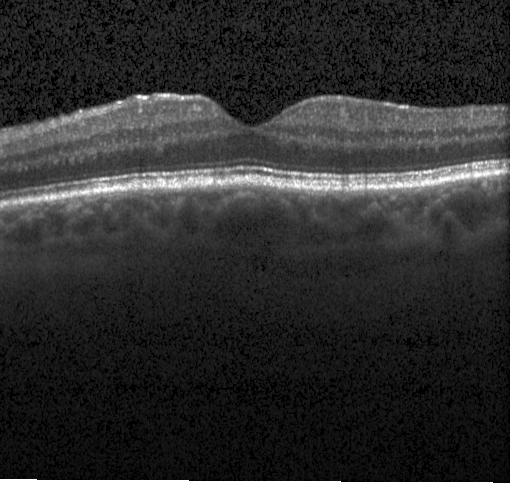
SD-OCT; Heidelberg Spectralis OCT system; optical coherence tomography scan
Finding: no choroidal neovascularization, diabetic macular edema, or drusen.